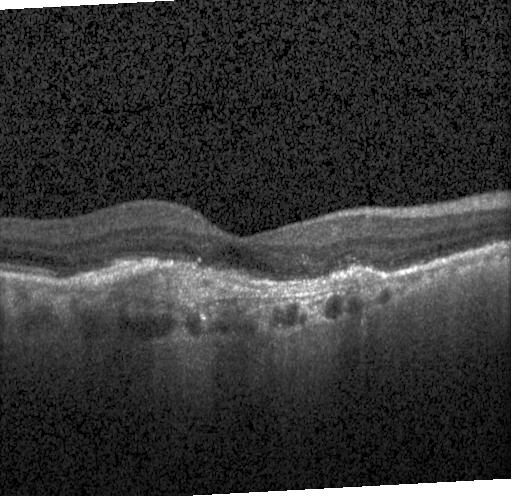 OCT B-scan — Assessment: choroidal neovascularization.